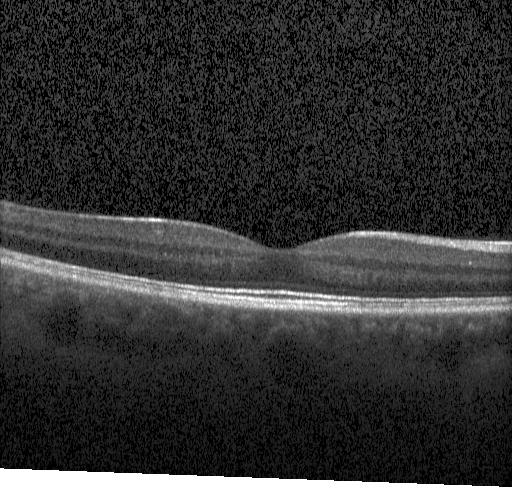
OCT B-scan, instrument: Heidelberg Spectralis, horizontal scan through the fovea. The scan shows neither choroidal neovascularization, diabetic macular edema, nor drusen.